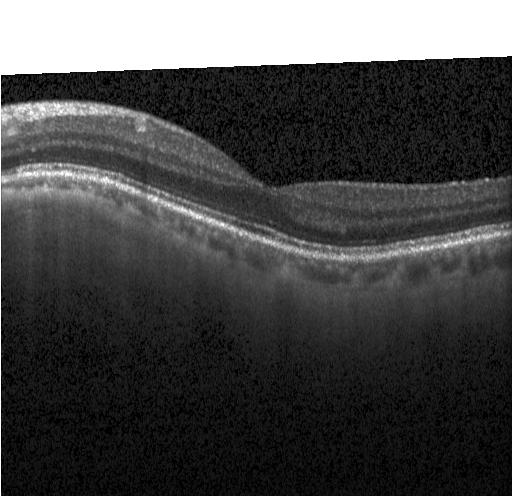
Optical coherence tomography B-scan · Heidelberg Spectralis OCT system.
The scan shows no choroidal neovascularization, diabetic macular edema, or drusen.